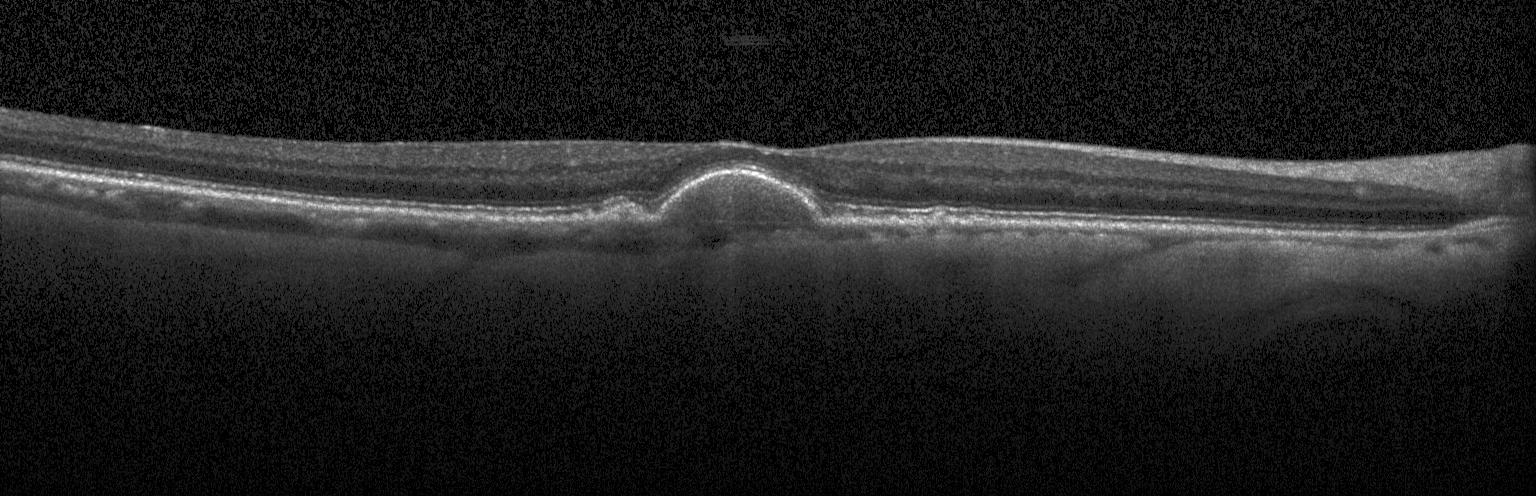 Diagnosis: a choroidal neovascular membrane.